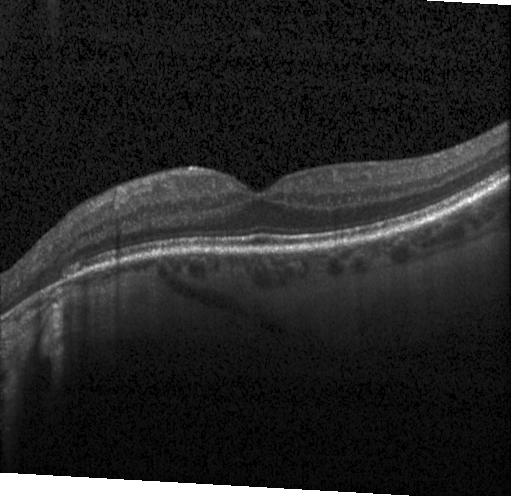

Heidelberg Spectralis; SD-OCT; fovea-centered; optical coherence tomography B-scan.
Dx: no choroidal neovascularization, diabetic macular edema, or drusen.